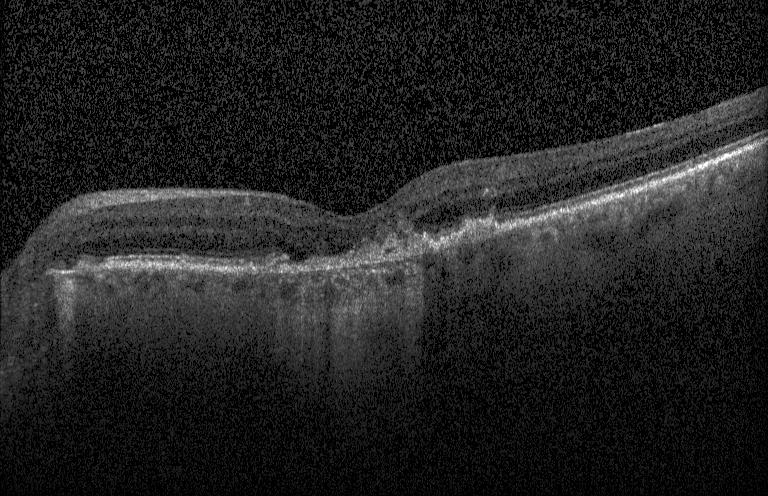

Spectral-domain optical coherence tomography; retinal OCT B-scan. The scan shows CNV.